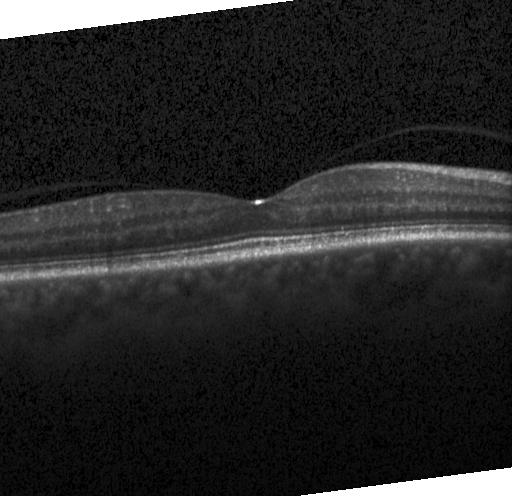
OCT B-scan showing no evidence of choroidal neovascularization, diabetic macular edema, or drusen.